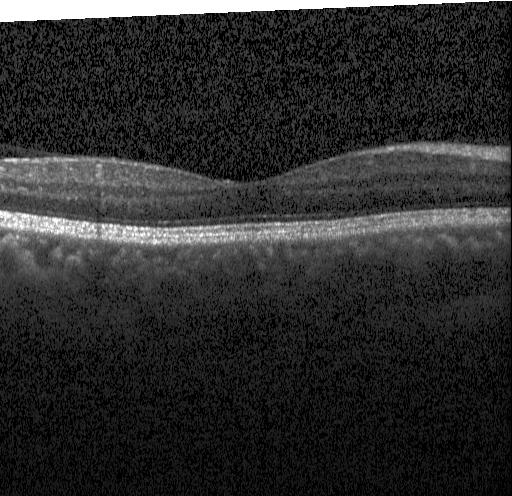
OCT finding: no choroidal neovascularization, diabetic macular edema, or drusen.